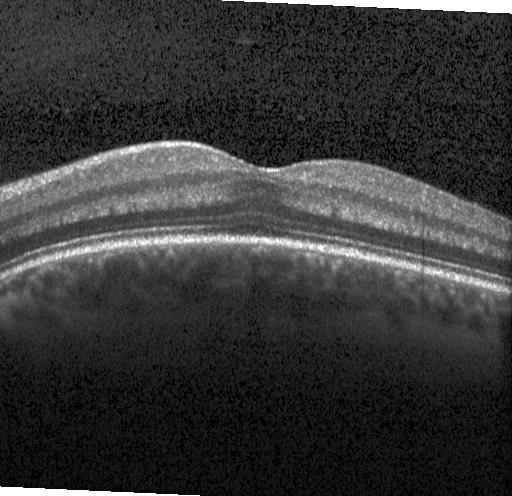 Diagnosis: no CNV, DME, or drusen.